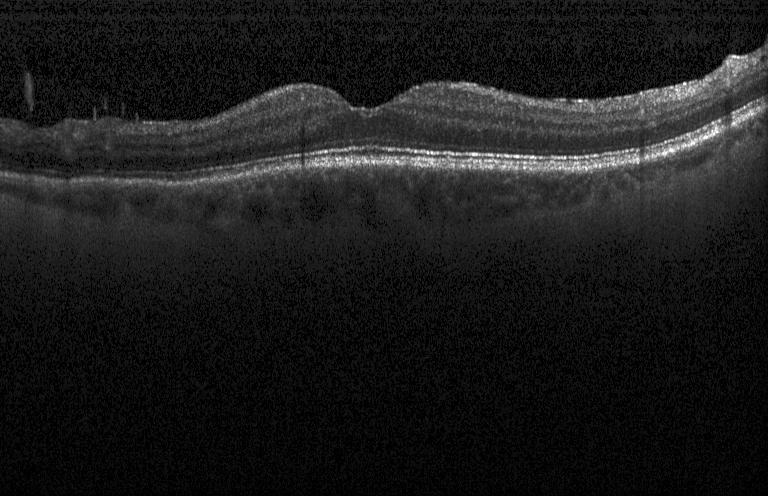 Finding: no evidence of choroidal neovascularization, diabetic macular edema, or drusen.